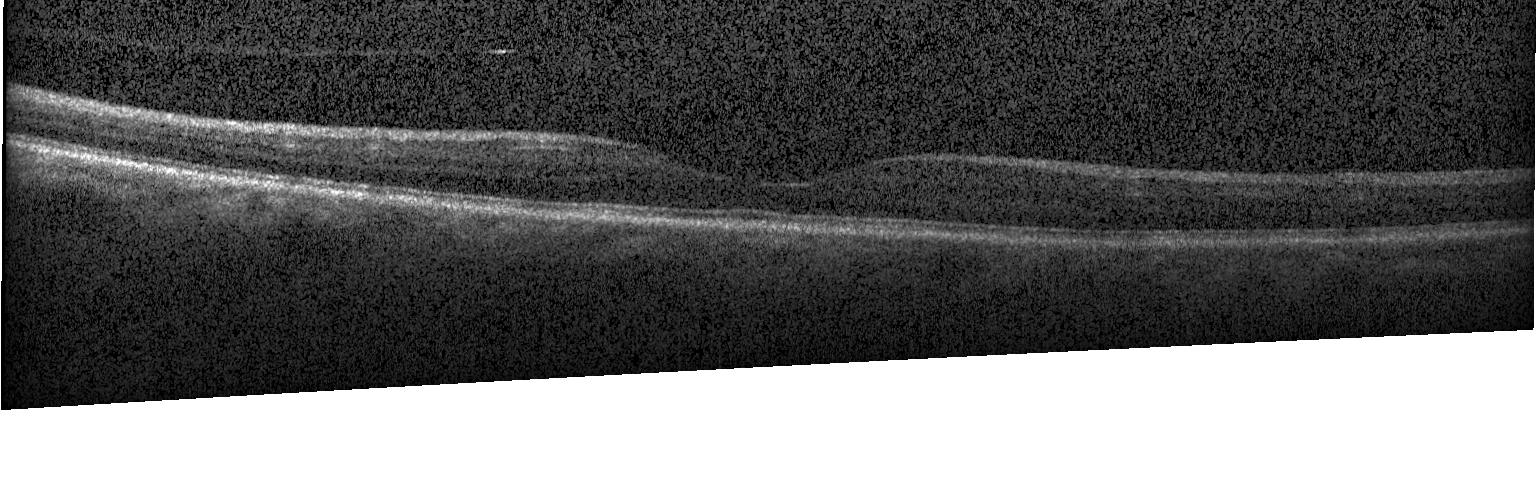

Acquired on a Heidelberg Spectralis, OCT line scan, through the macula.
Macular OCT: no choroidal neovascularization, no diabetic macular edema, and no drusen.